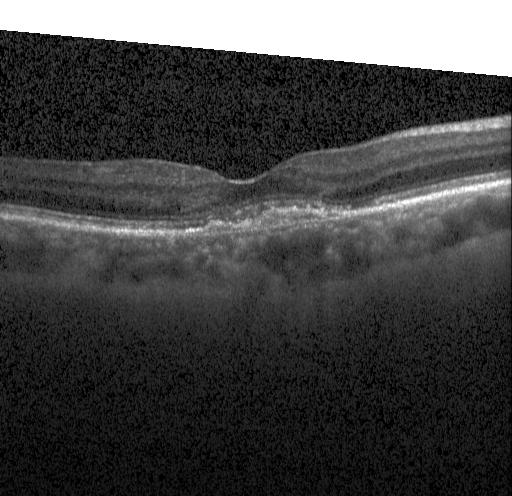
Spectral-domain optical coherence tomography. OCT B-scan. Heidelberg Spectralis OCT system — Finding: choroidal neovascularization (CNV).